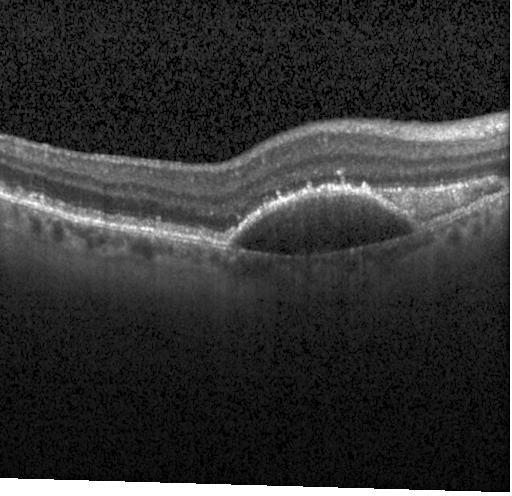 OCT B-scan. Centered on the fovea. Spectral-domain OCT. Heidelberg Spectralis OCT system.
This B-scan demonstrates a choroidal neovascular membrane.